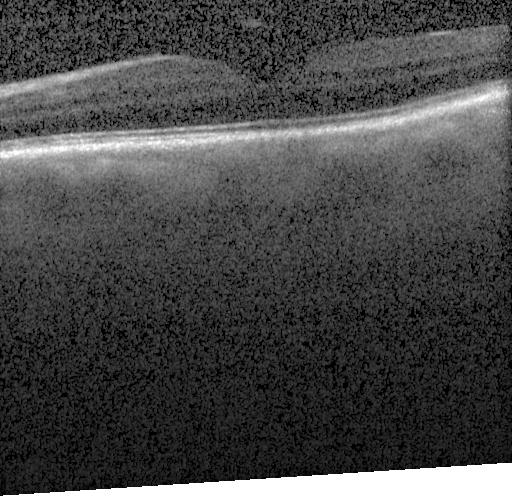
No choroidal neovascularization, no diabetic macular edema, and no drusen.